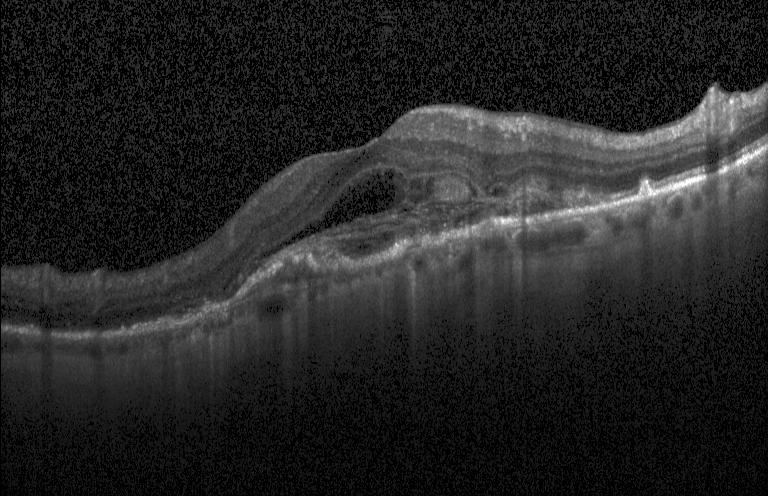
Macular OCT demonstrating choroidal neovascularization.